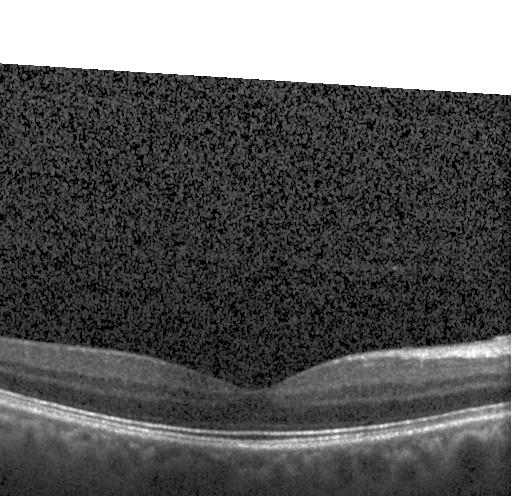 Macular OCT demonstrating no CNV, no DME, and no drusen.